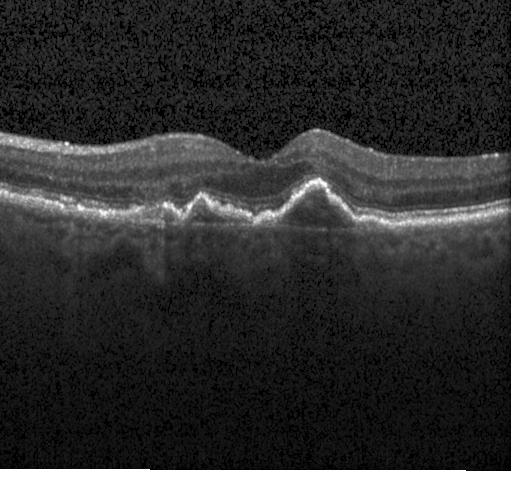 Instrument: Heidelberg Spectralis, macular scan, retinal OCT cross-section. Finding: a choroidal neovascular membrane.